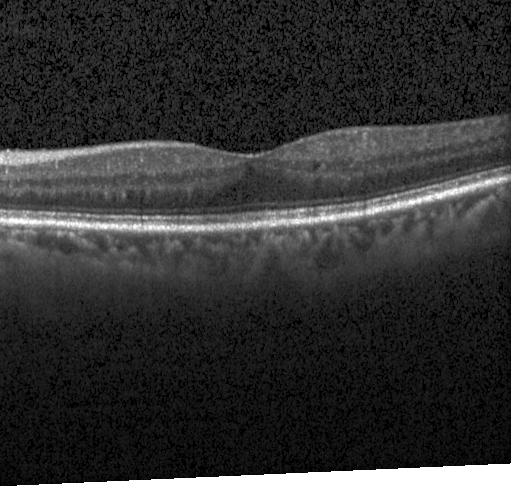 OCT B-scan, centered on the fovea
Macular OCT: no choroidal neovascularization, no diabetic macular edema, and no drusen.